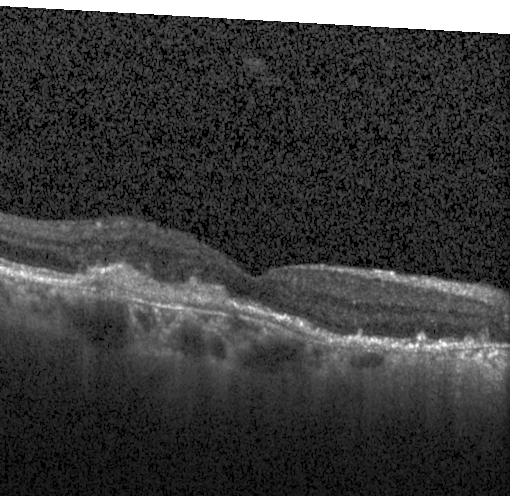
Retinal OCT B-scan. Macular OCT: CNV.